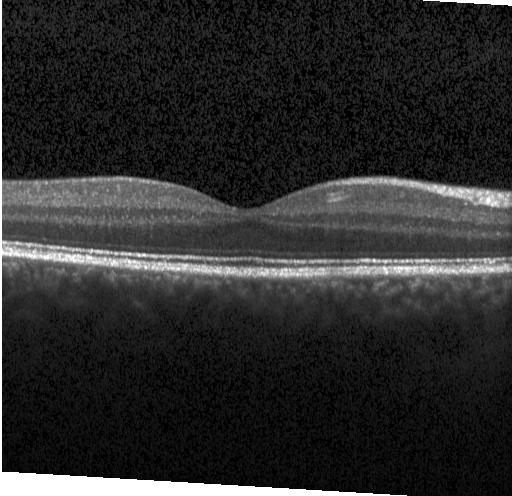

The scan shows no CNV, DME, or drusen.